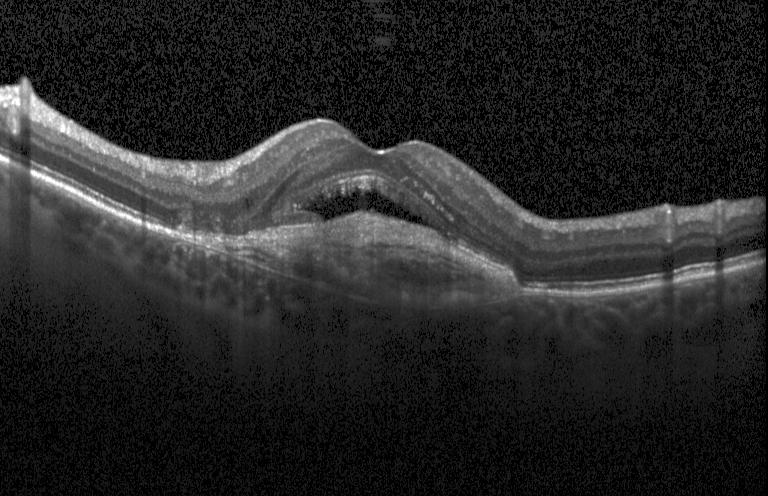 Optical coherence tomography B-scan · SD-OCT · instrument: Heidelberg Spectralis
Macular OCT: CNV.